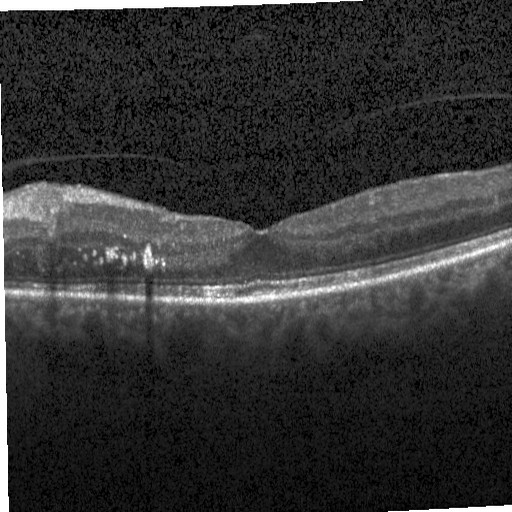
Diabetic macular edema.